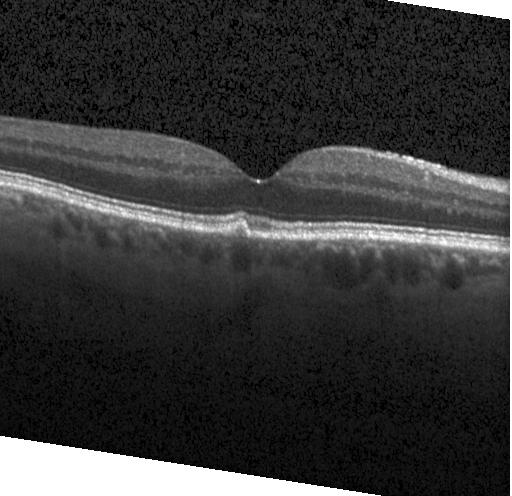 This B-scan demonstrates multiple drusen.